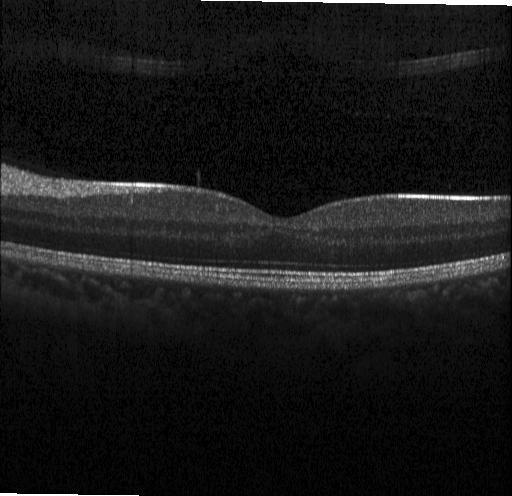

Impression: no choroidal neovascularization, no diabetic macular edema, and no drusen.